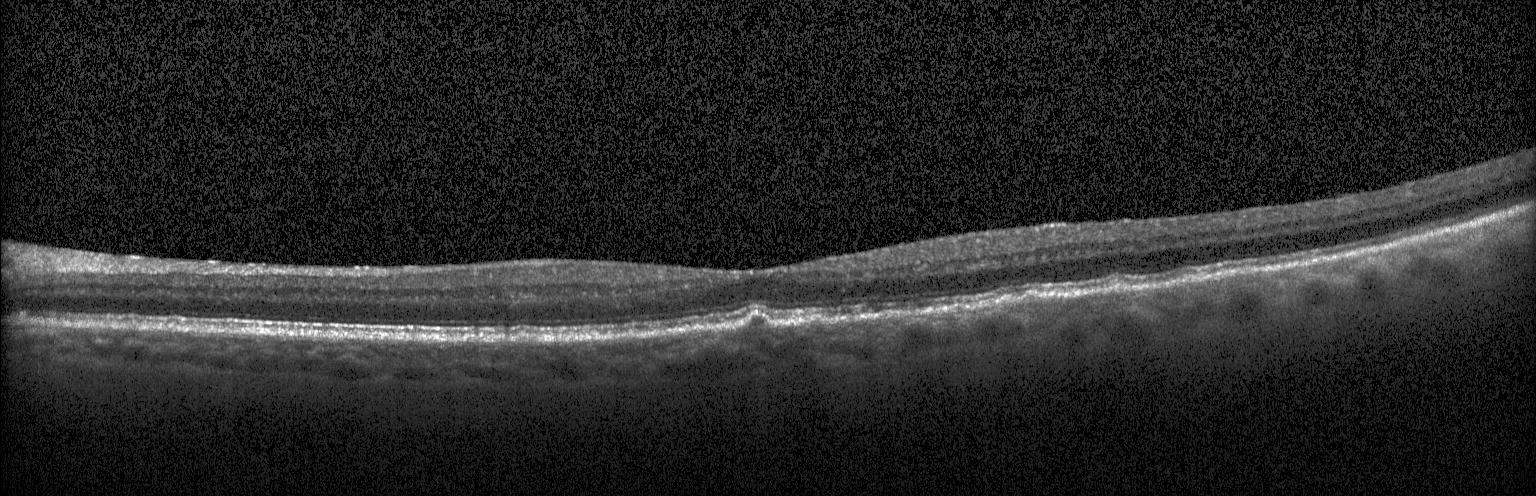 Assessment: multiple drusen.